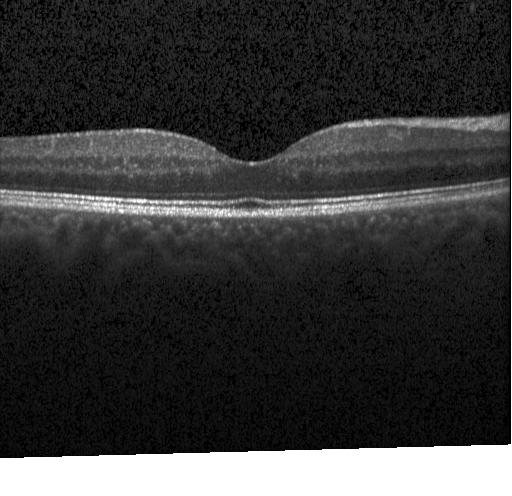

Dx: no evidence of choroidal neovascularization, diabetic macular edema, or drusen.